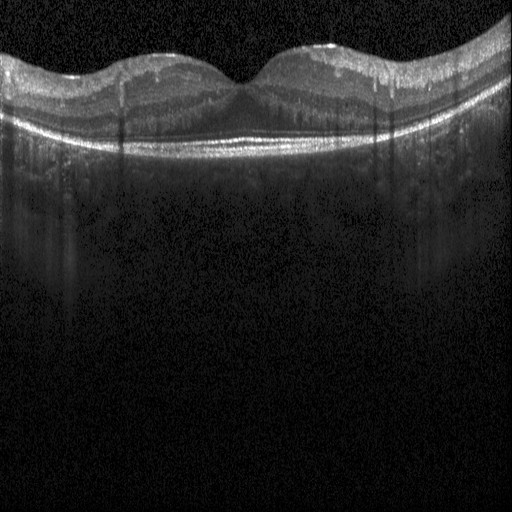
OCT B-scan showing diabetic macular edema.